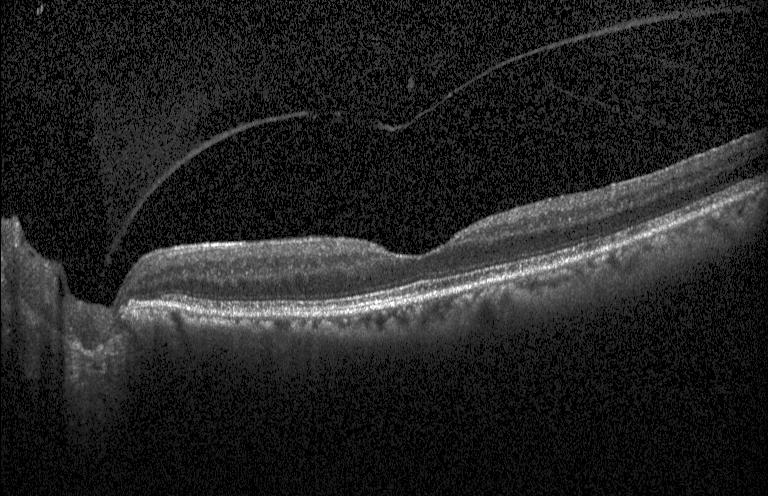

Spectral-domain OCT, optical coherence tomography B-scan, Heidelberg Spectralis OCT system, horizontal scan through the fovea
The scan shows neither choroidal neovascularization, diabetic macular edema, nor drusen.